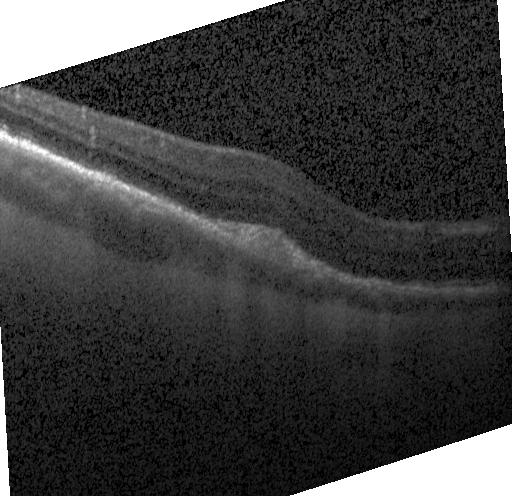
A choroidal neovascular membrane.